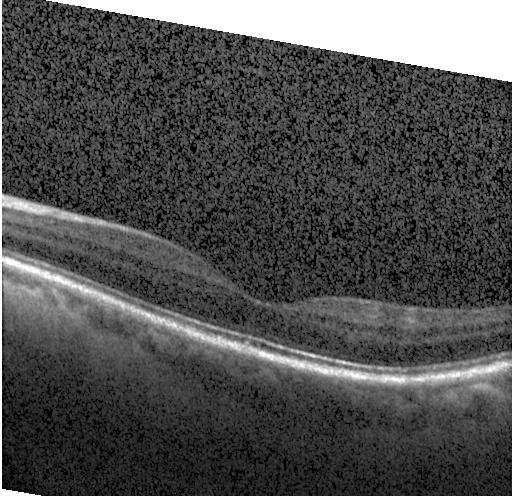
Acquired on a Heidelberg Spectralis. SD-OCT. Retinal OCT B-scan
No CNV, DME, or drusen.